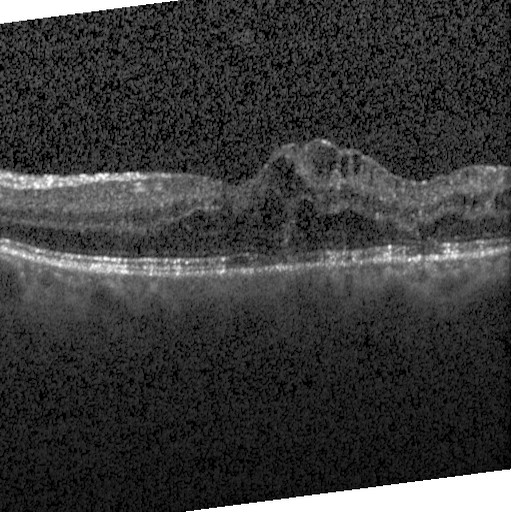 Spectral-domain OCT. Heidelberg Spectralis OCT system. Macular scan. Retinal OCT cross-section. This B-scan demonstrates DME.